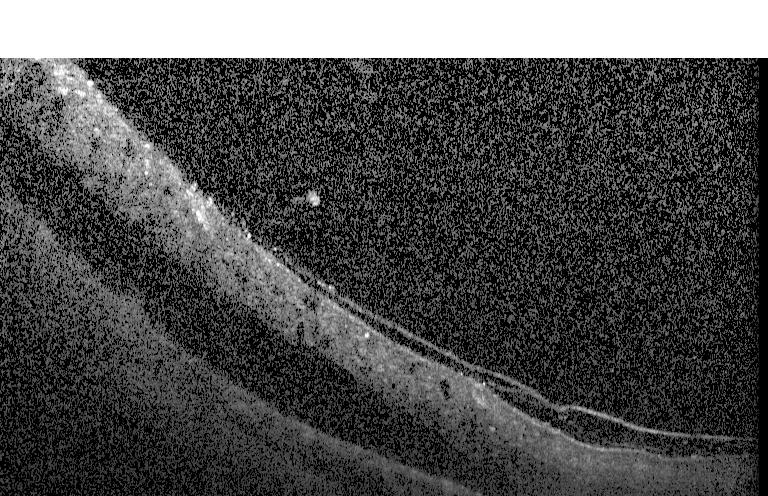 Finding: DME.